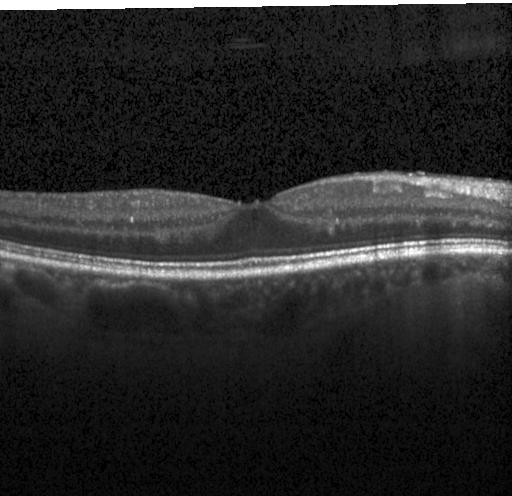 Assessment: no choroidal neovascularization, diabetic macular edema, or drusen.